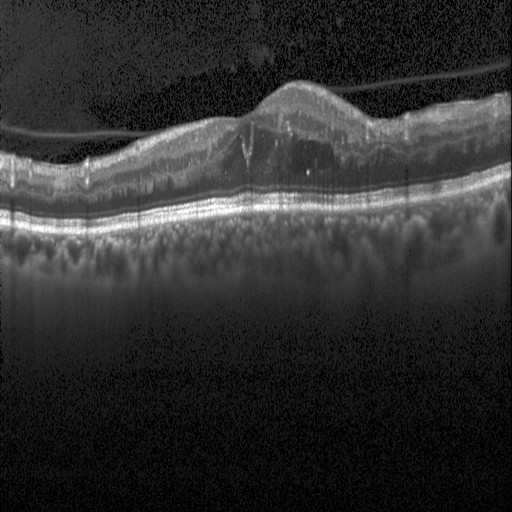

OCT finding: diabetic macular edema.